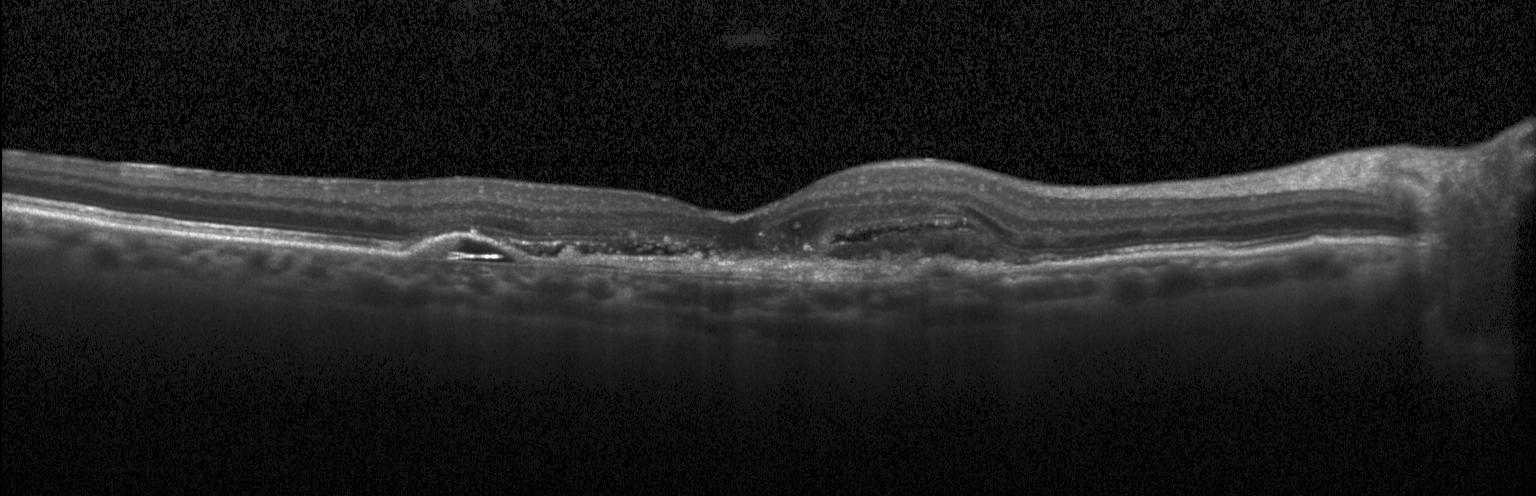

OCT finding: choroidal neovascularization.